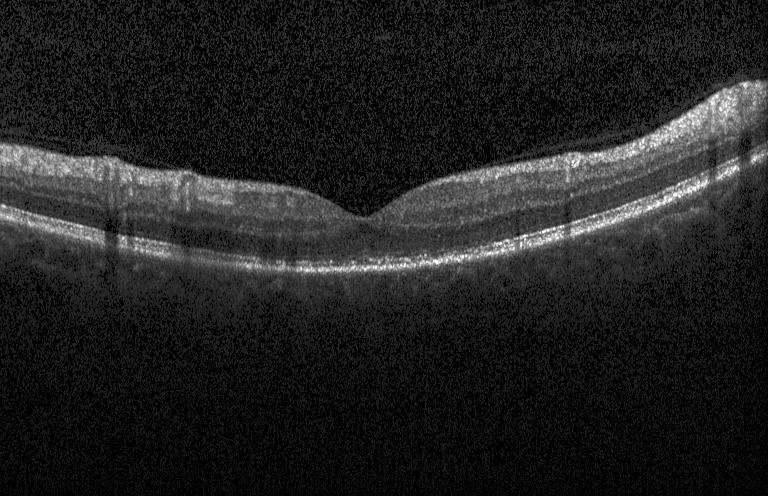

OCT line scan · instrument: Heidelberg Spectralis · macular scan · SD-OCT. Neither choroidal neovascularization, diabetic macular edema, nor drusen.